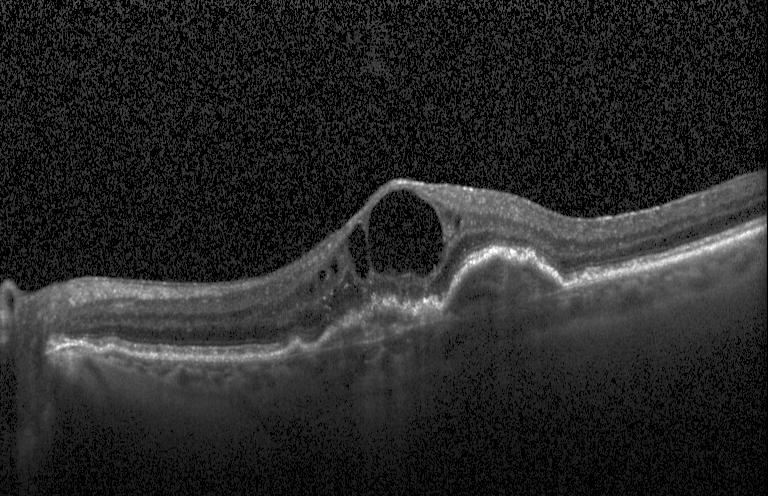
Retinal OCT cross-section — Diagnosis: choroidal neovascularization.